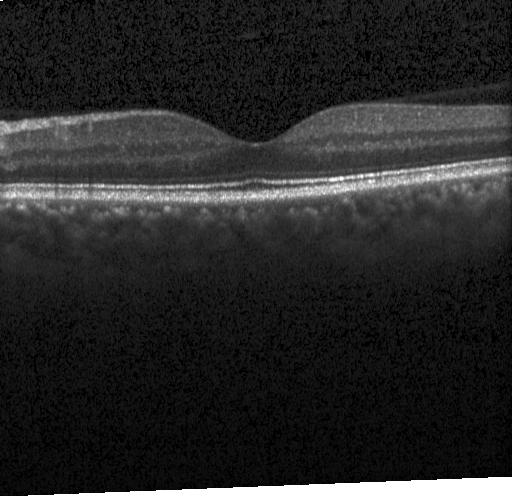
Fovea-centered, optical coherence tomography scan, Heidelberg Spectralis
Impression: neither choroidal neovascularization, diabetic macular edema, nor drusen.